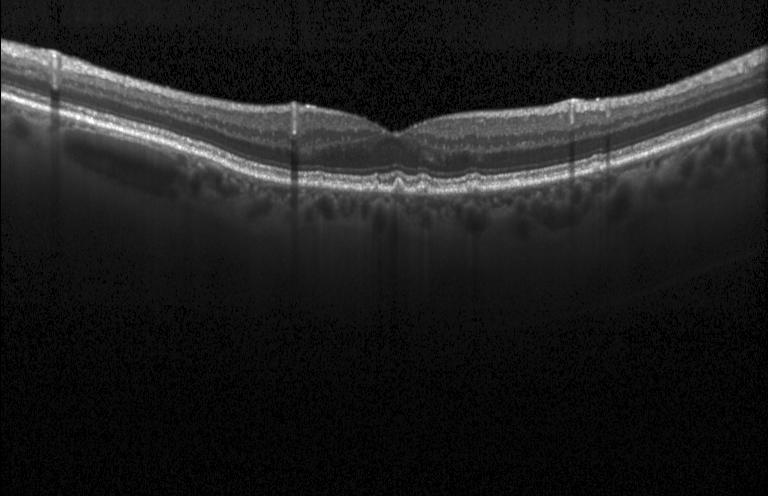
Finding: multiple drusen.